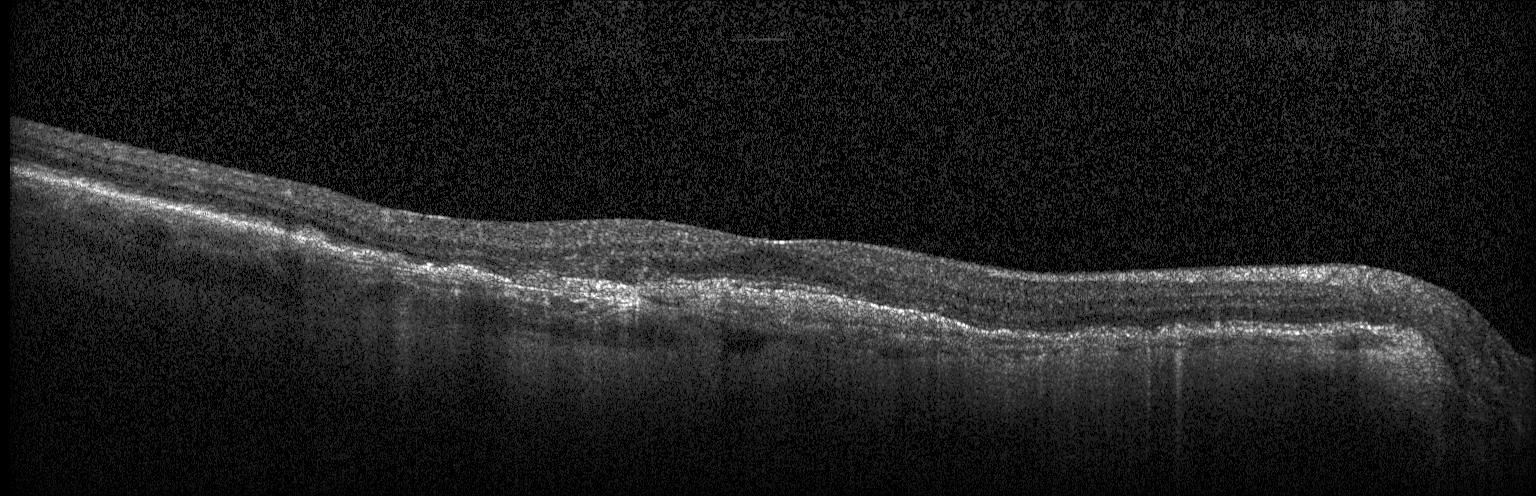

Diagnosis: choroidal neovascularization (CNV).